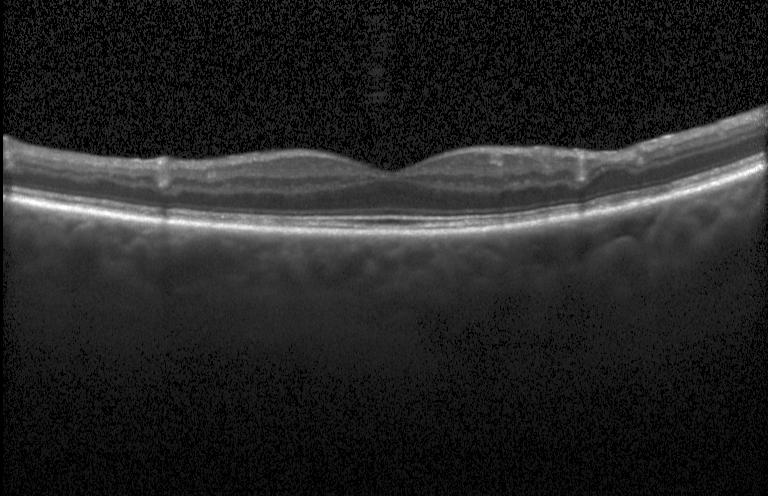

Diagnosis: no CNV, DME, or drusen.